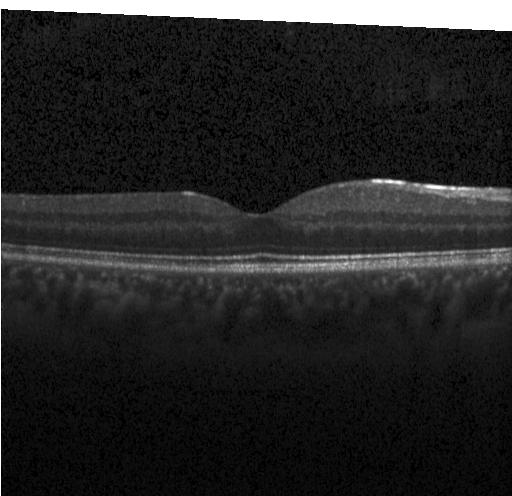
Optical coherence tomography B-scan — Dx: no choroidal neovascularization, diabetic macular edema, or drusen.